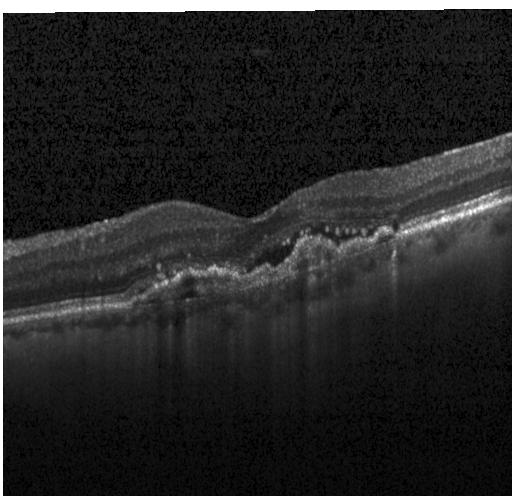

Retinal OCT B-scan. Acquired on a Heidelberg Spectralis. Macular scan. Spectral-domain OCT — Diagnosis: CNV.